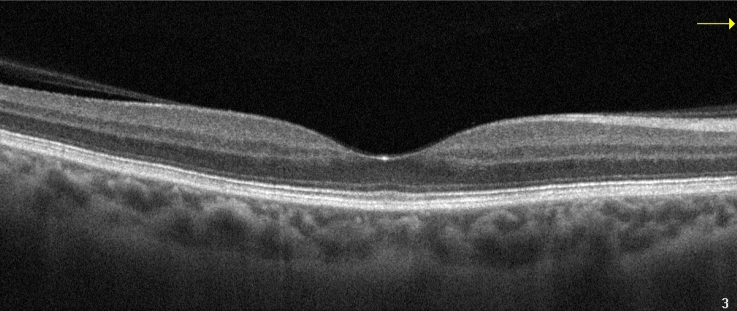 Macular OCT demonstrating no AMD, DME, ERM, RAO, RVO, or VID.